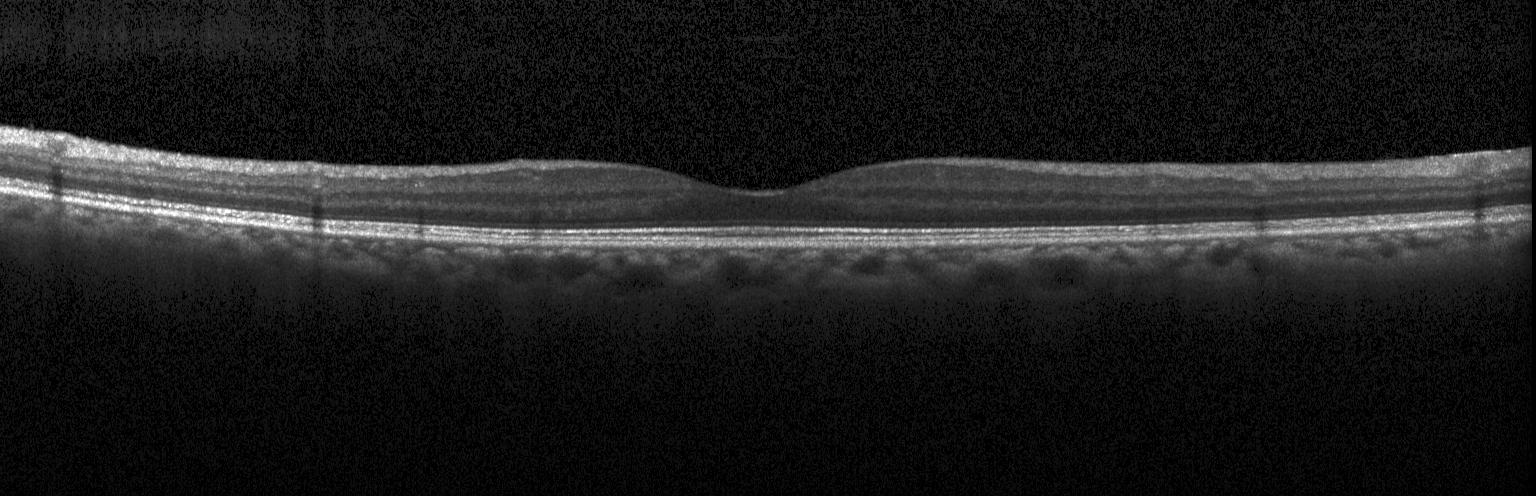

OCT scan showing neither choroidal neovascularization, diabetic macular edema, nor drusen.